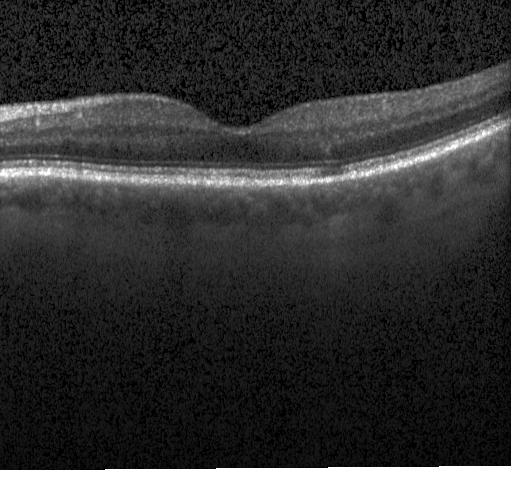

Retinal OCT B-scan. Spectral-domain OCT. Acquired on a Heidelberg Spectralis
Dx: neither CNV, DME, nor drusen.